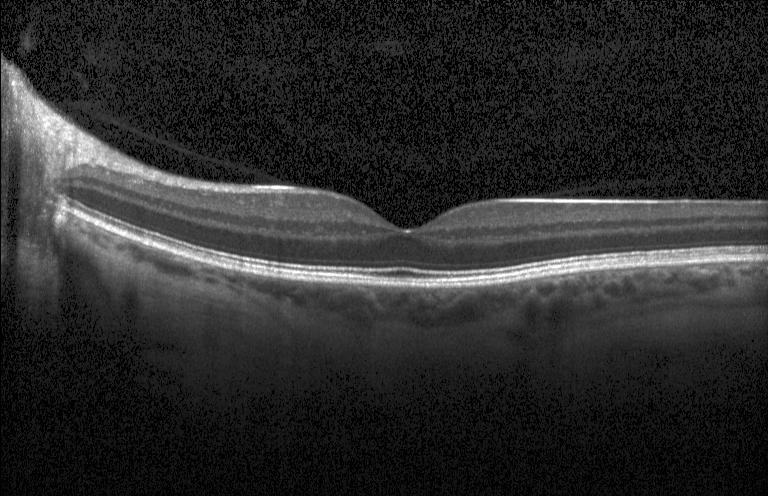

Optical coherence tomography scan. Acquired on a Heidelberg Spectralis. Spectral-domain optical coherence tomography. Fovea-centered. Diagnosis: no evidence of choroidal neovascularization, diabetic macular edema, or drusen.